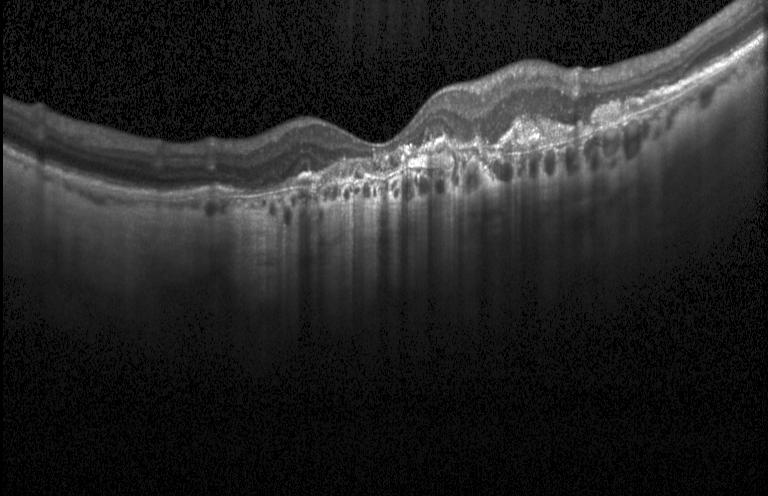

Centered on the fovea · optical coherence tomography B-scan
Impression: a choroidal neovascular membrane.